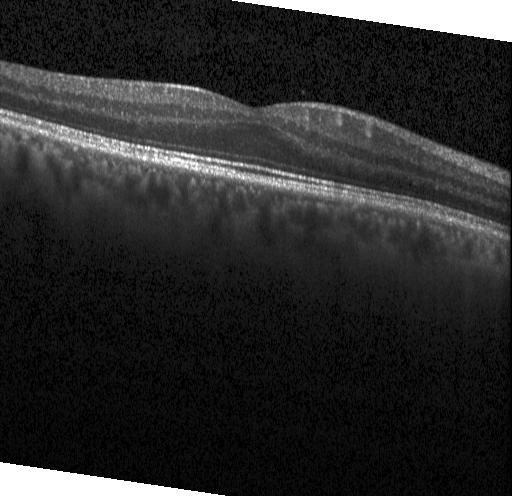
Impression: no evidence of choroidal neovascularization, diabetic macular edema, or drusen.